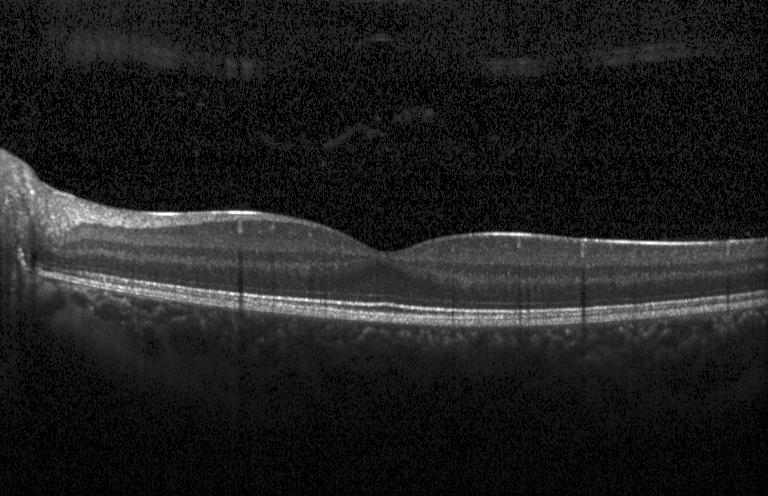

Spectral-domain OCT B-scan: no choroidal neovascularization, no diabetic macular edema, and no drusen.